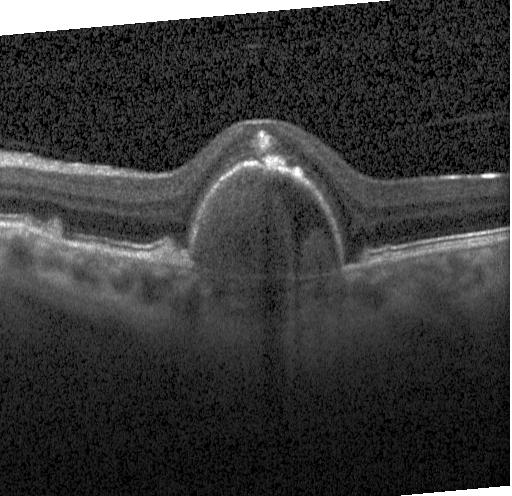

Horizontal scan through the fovea, optical coherence tomography scan, Heidelberg Spectralis OCT system
Finding: a choroidal neovascular membrane.